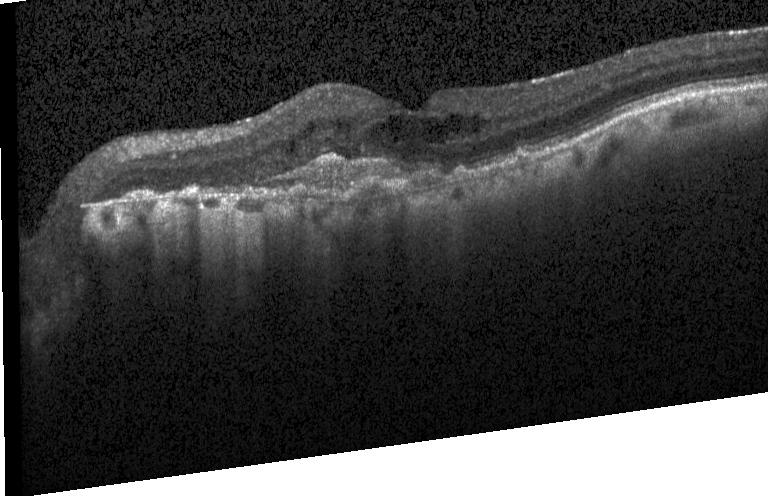

Diagnosis: choroidal neovascularization.